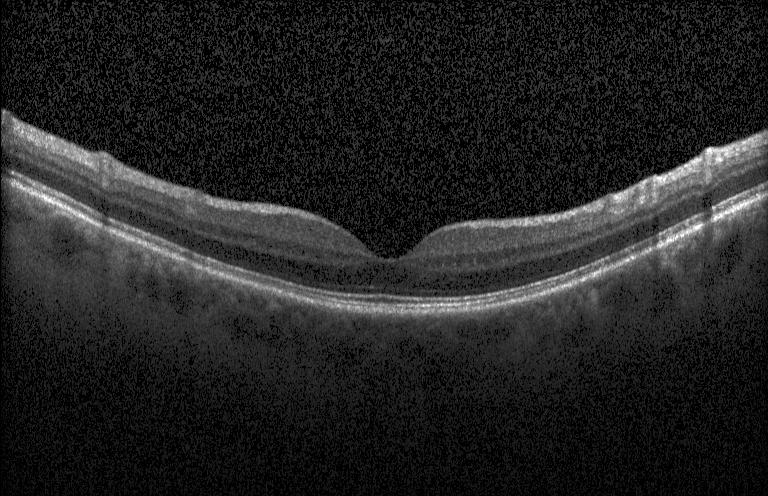

No choroidal neovascularization, diabetic macular edema, or drusen.